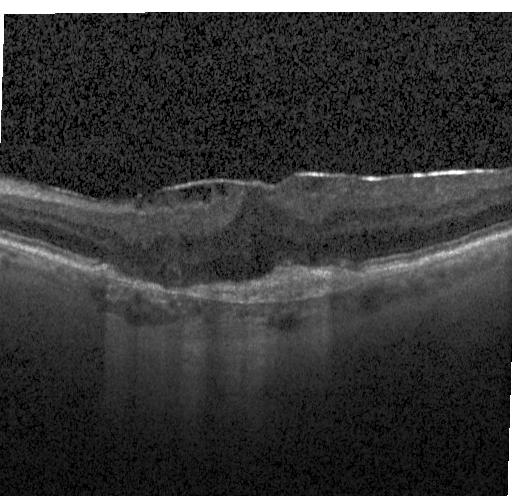

Retinal OCT B-scan; SD-OCT. Diagnosis: a choroidal neovascular membrane.